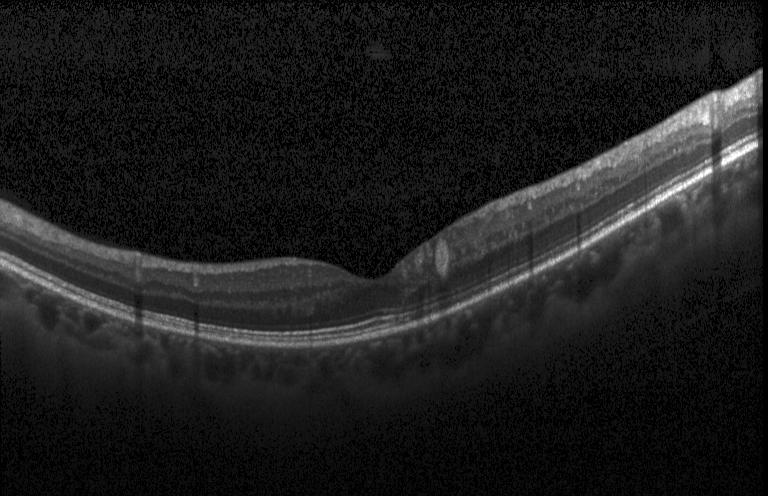
Dx: no choroidal neovascularization, diabetic macular edema, or drusen.